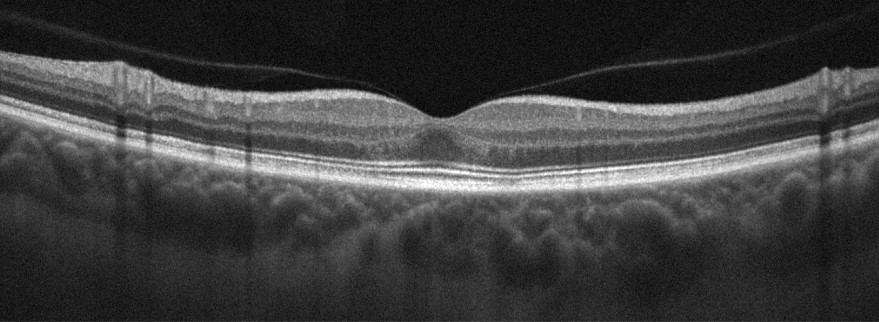

Through the macula, Optovue Avanti RTVue XR, OCT line scan — Impression: no AMD, DME, ERM, RAO, RVO, or VID.